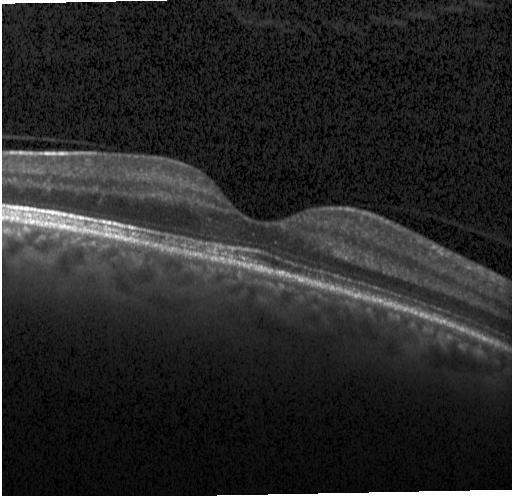
Spectral-domain OCT. OCT line scan. Heidelberg Spectralis OCT system.
OCT finding: neither choroidal neovascularization, diabetic macular edema, nor drusen.